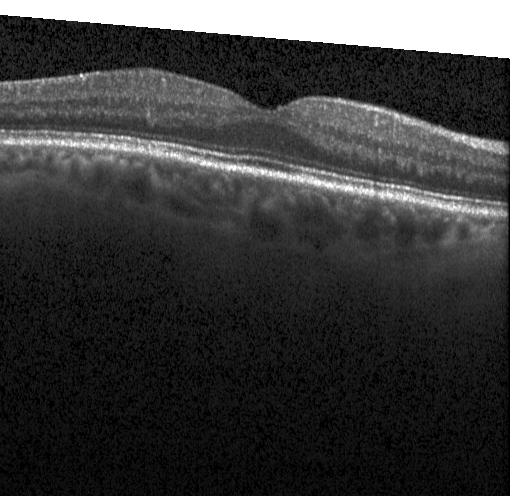 Heidelberg Spectralis OCT system · optical coherence tomography B-scan
The scan shows no CNV, DME, or drusen.